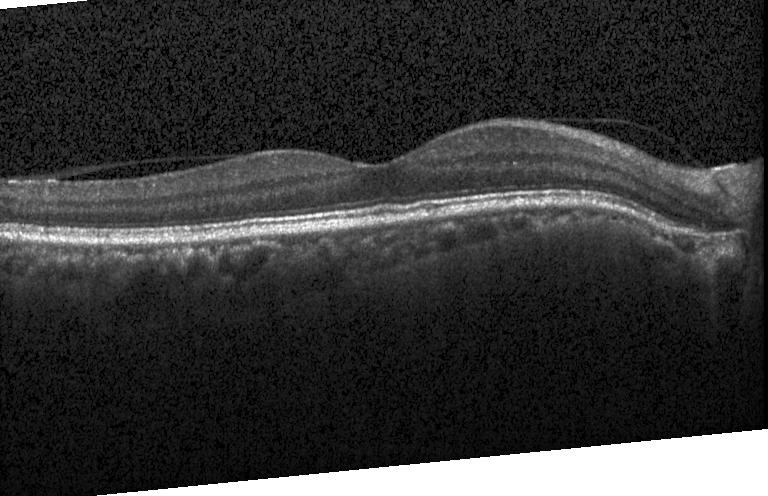
Instrument: Heidelberg Spectralis; retinal OCT cross-section.
Finding: no evidence of CNV, DME, or drusen.